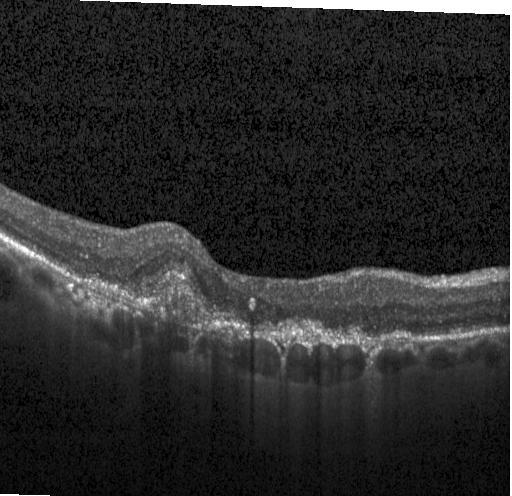
Centered on the fovea · OCT line scan · spectral-domain OCT · acquired on a Heidelberg Spectralis.
Finding: a choroidal neovascular membrane.